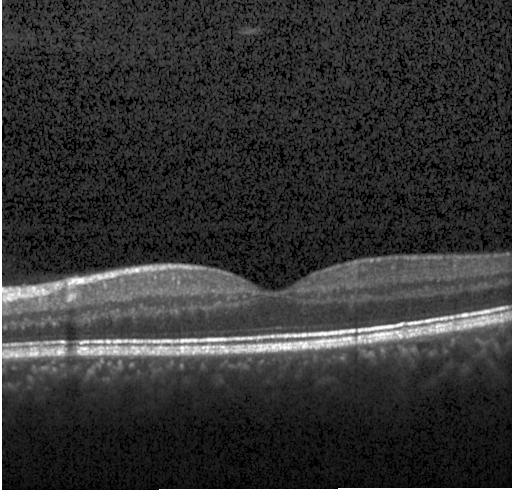
Finding: no choroidal neovascularization, diabetic macular edema, or drusen.